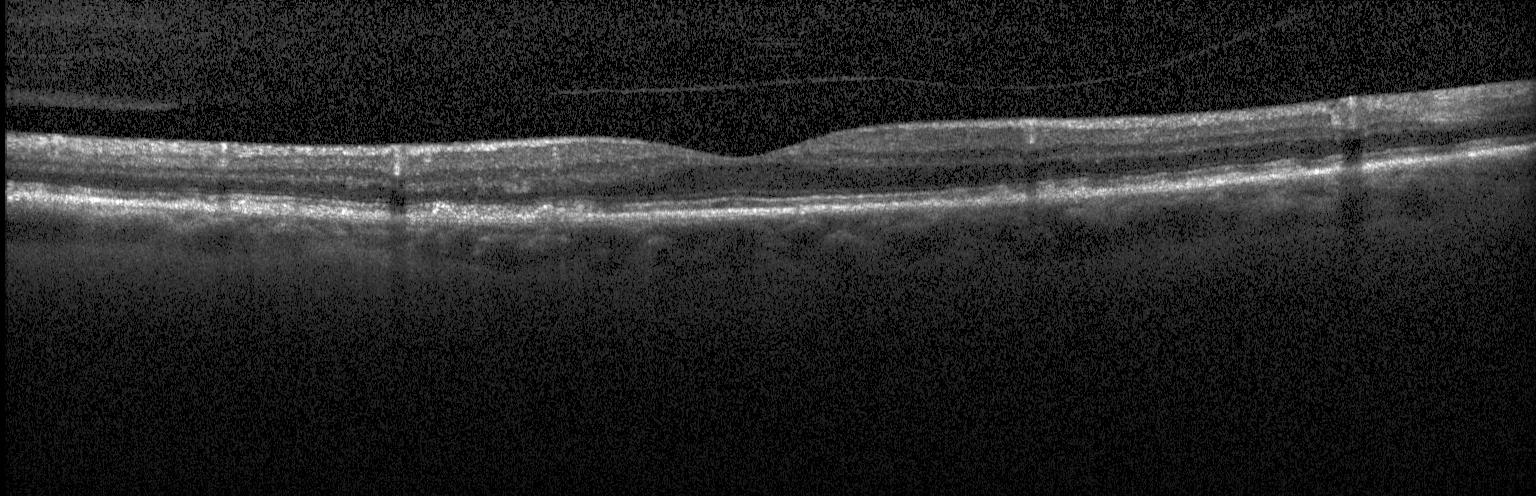 Impression: multiple drusen.